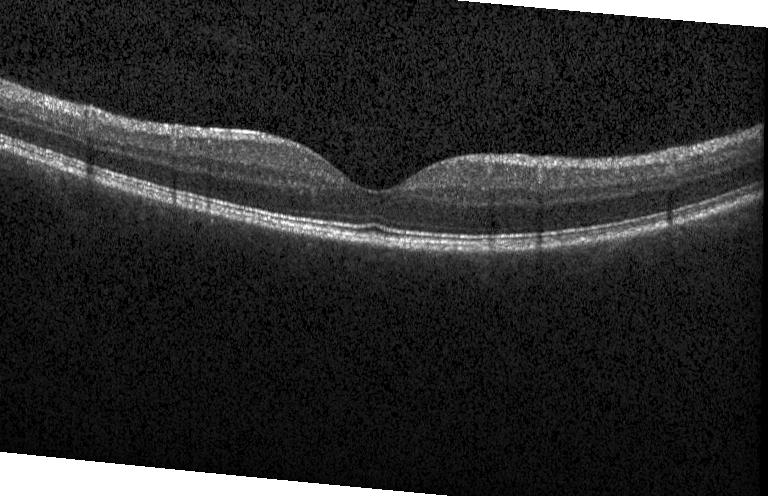
Spectral-domain OCT · centered on the fovea · optical coherence tomography B-scan — Diagnosis: no choroidal neovascularization, no diabetic macular edema, and no drusen.